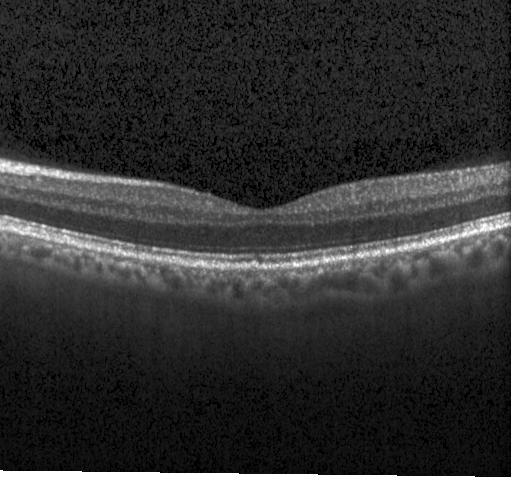

OCT B-scan showing no choroidal neovascularization, no diabetic macular edema, and no drusen.